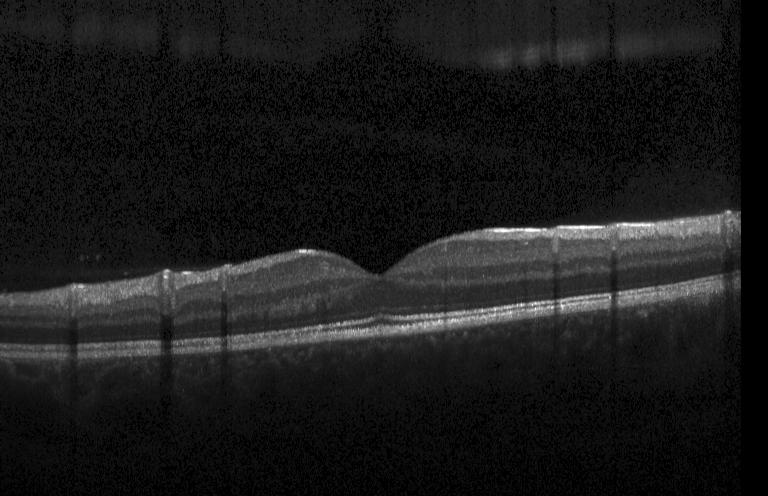 OCT scan showing no CNV, no DME, and no drusen.